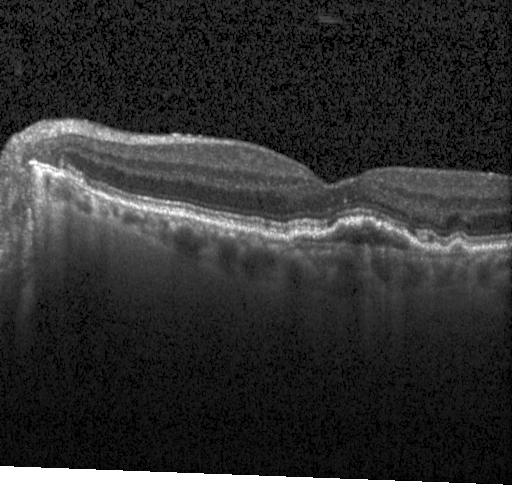
Retinal OCT cross-section showing choroidal neovascularization.